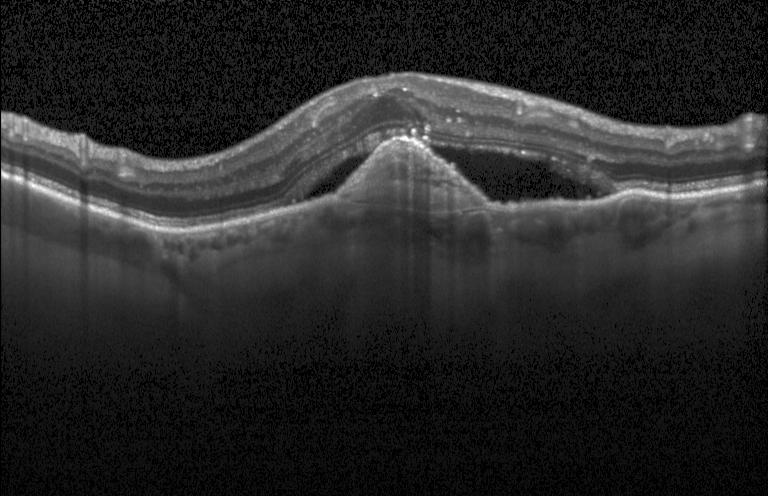

A choroidal neovascular membrane.